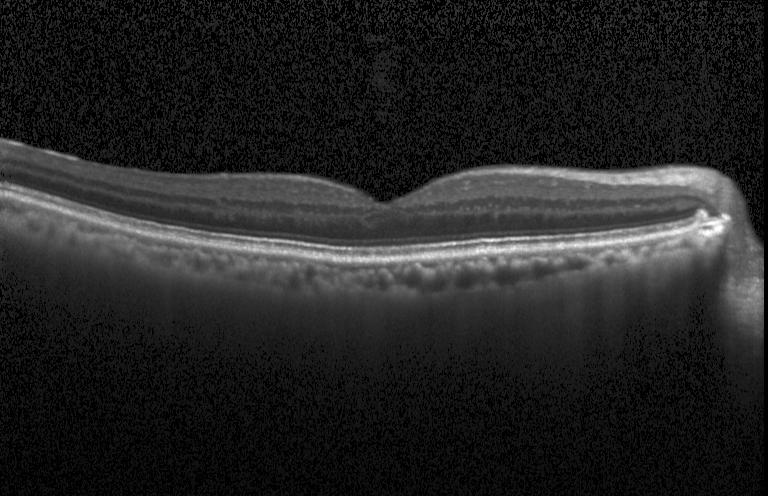
Finding: no evidence of choroidal neovascularization, diabetic macular edema, or drusen.